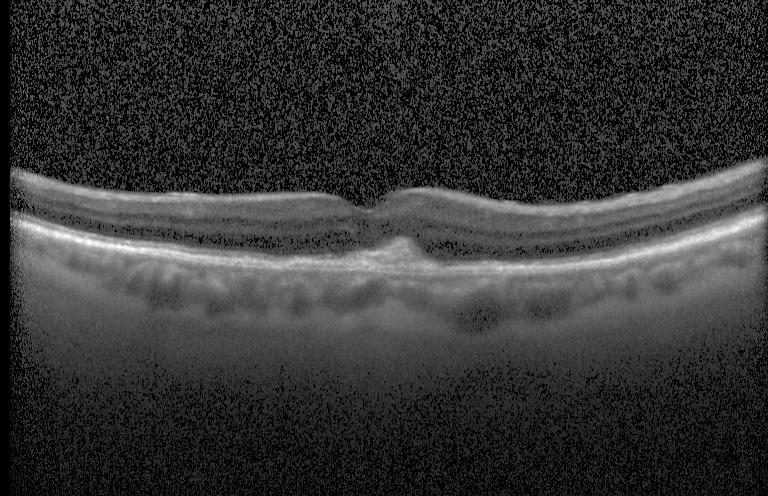 The scan shows a choroidal neovascular membrane.